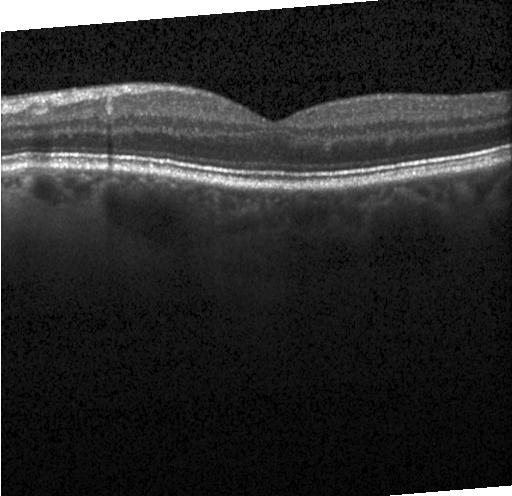 Acquired on a Heidelberg Spectralis · OCT line scan · spectral-domain OCT. Diagnosis: no choroidal neovascularization, diabetic macular edema, or drusen.